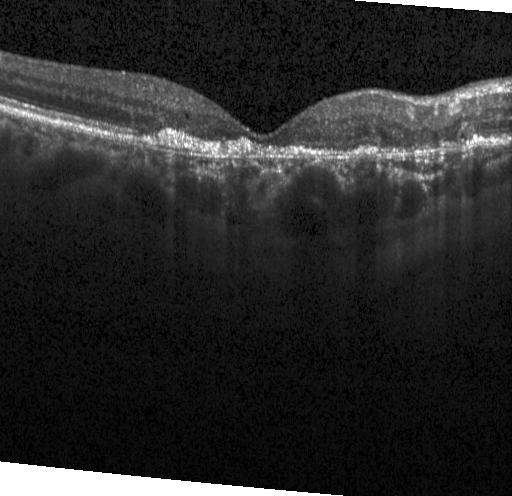 Spectral-domain optical coherence tomography; through the macula; optical coherence tomography B-scan. Diagnosis: a choroidal neovascular membrane.